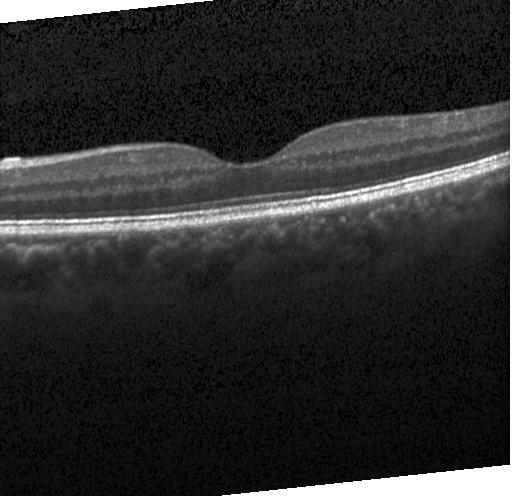
Retinal OCT cross-section showing neither CNV, DME, nor drusen.